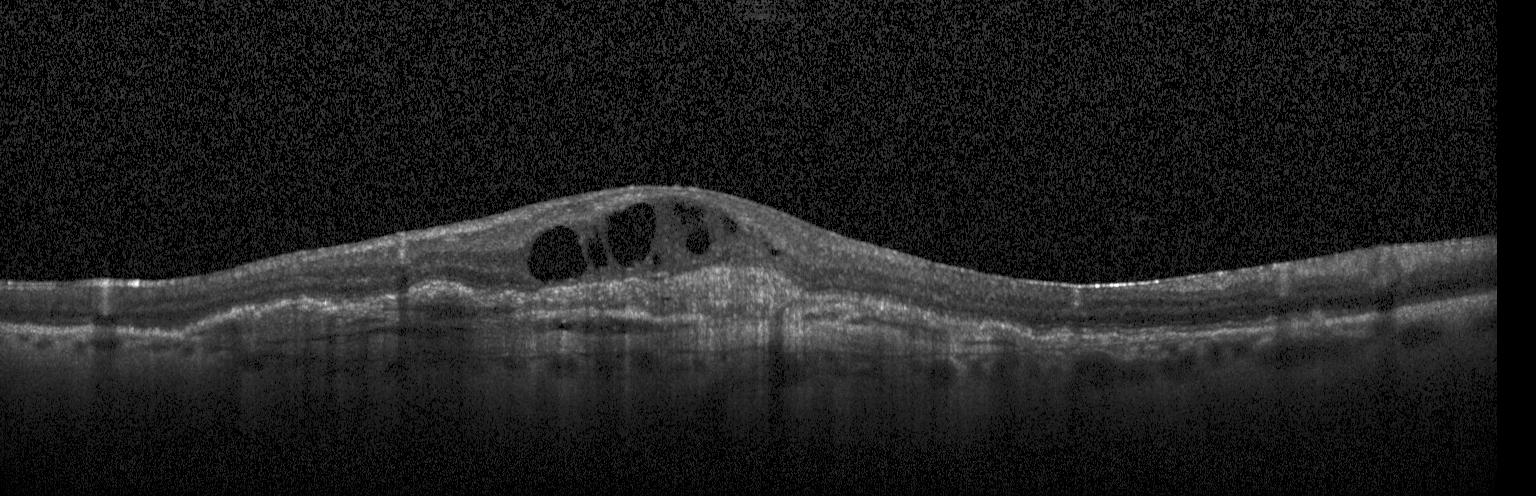 OCT line scan. Macular OCT: a choroidal neovascular membrane.